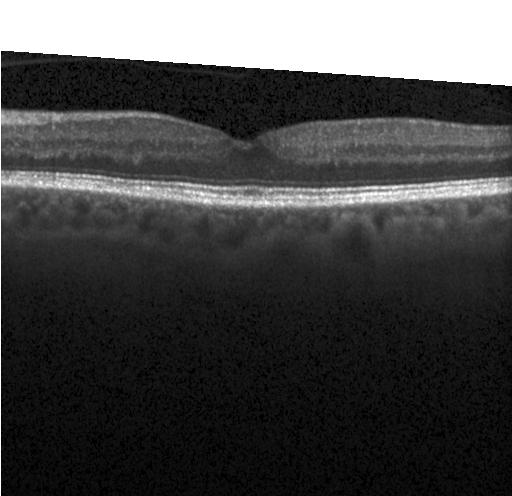 Diagnosis: no choroidal neovascularization, no diabetic macular edema, and no drusen.